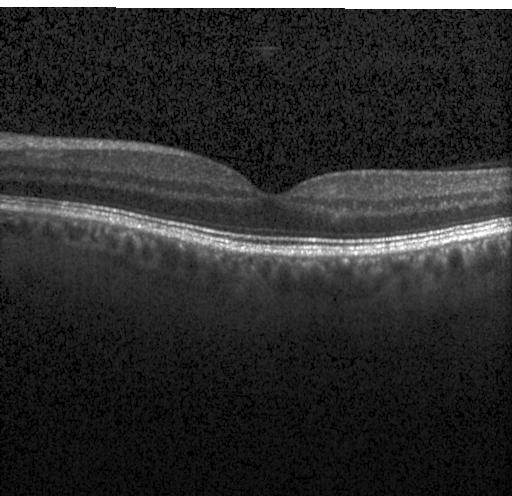

Diagnosis: no CNV, DME, or drusen.